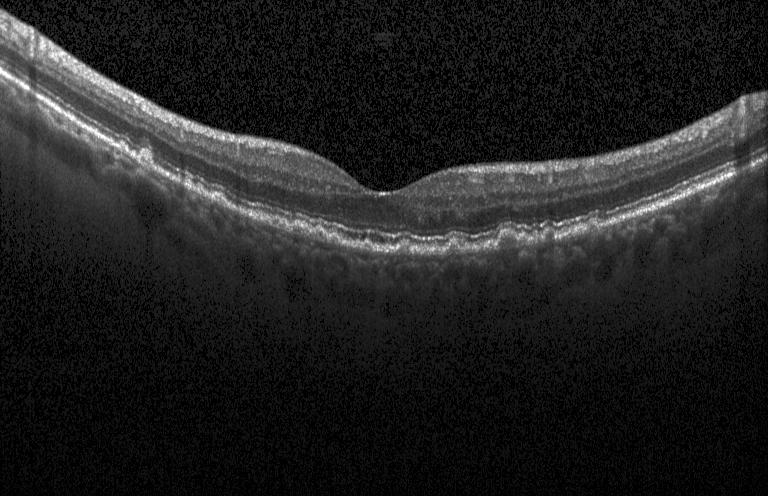
Fovea-centered; acquired on a Heidelberg Spectralis; optical coherence tomography scan. Finding: sub-RPE drusenoid deposits.